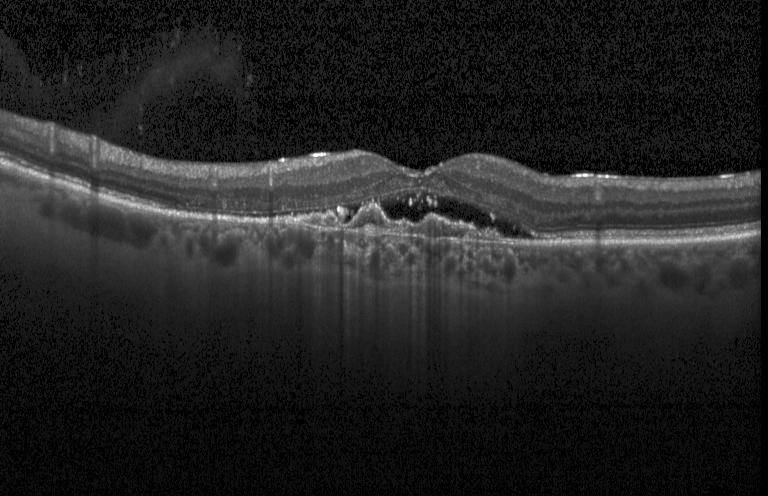 Optical coherence tomography B-scan. Finding: a choroidal neovascular membrane.